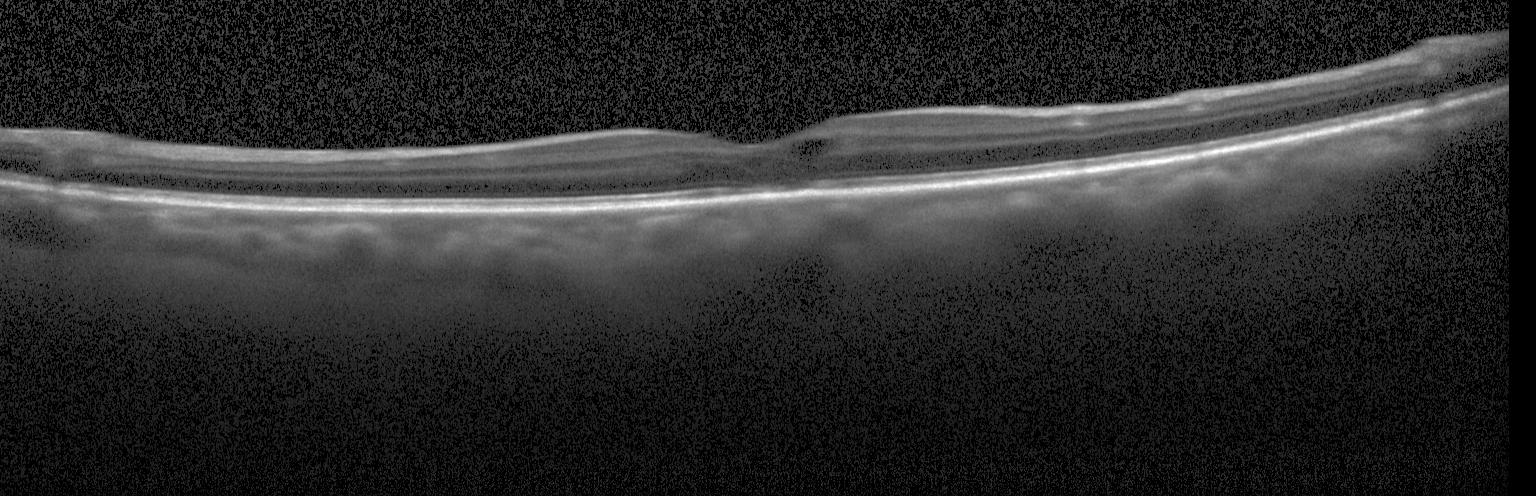 Retinal OCT B-scan
This B-scan demonstrates DME.